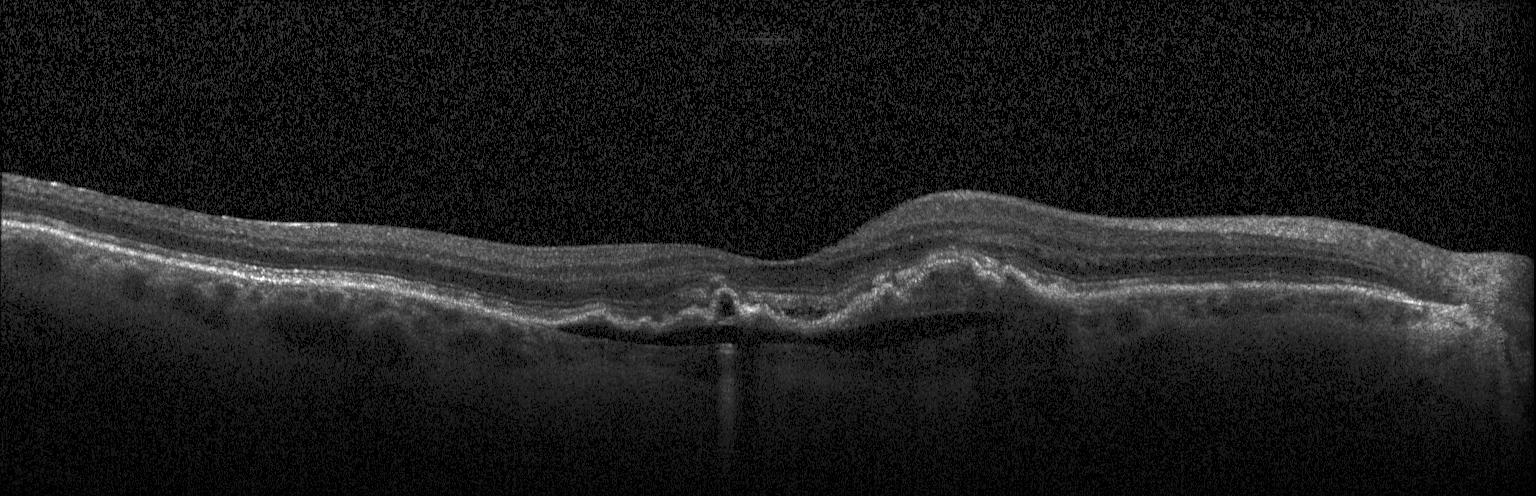 Diagnosis: choroidal neovascularization.